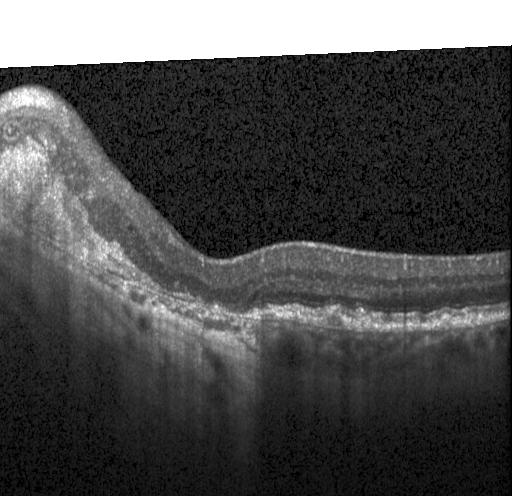
Horizontal scan through the fovea · spectral-domain OCT · instrument: Heidelberg Spectralis · retinal OCT B-scan — The scan shows a choroidal neovascular membrane.